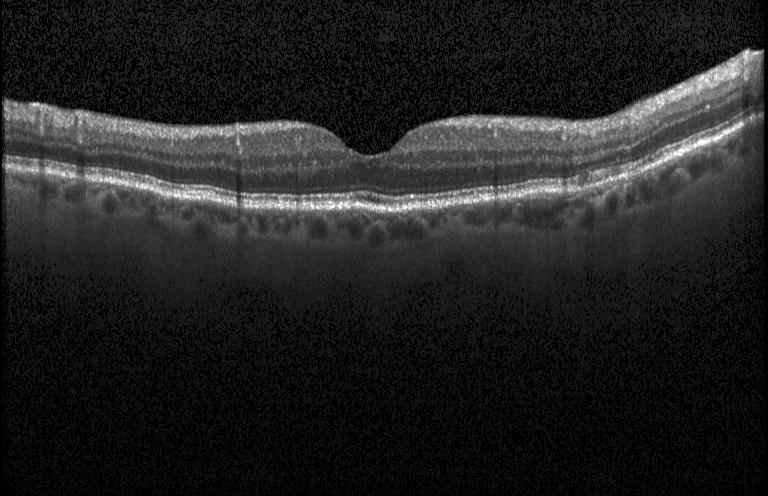

Macular scan; optical coherence tomography scan.
The scan shows no choroidal neovascularization, diabetic macular edema, or drusen.